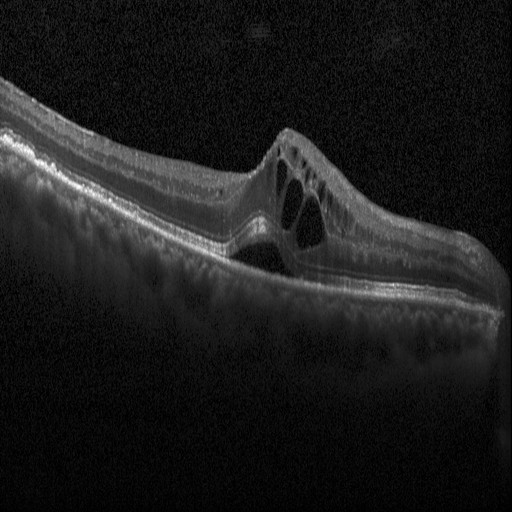 OCT B-scan.
Diagnosis: DME.